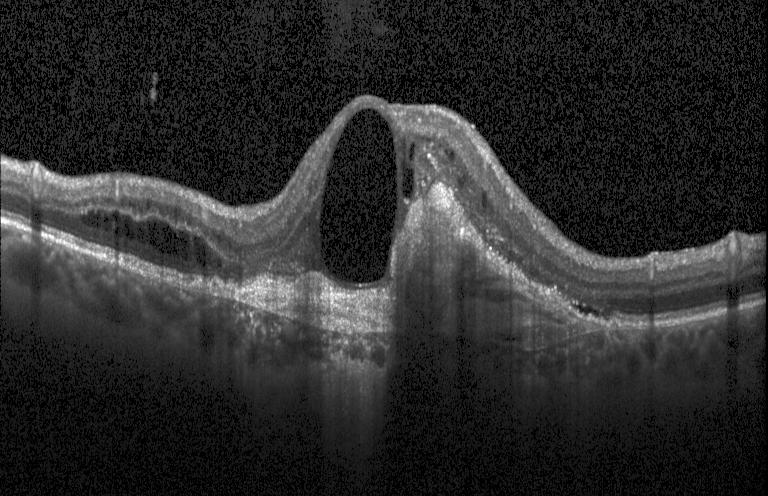

Diagnosis: CNV.